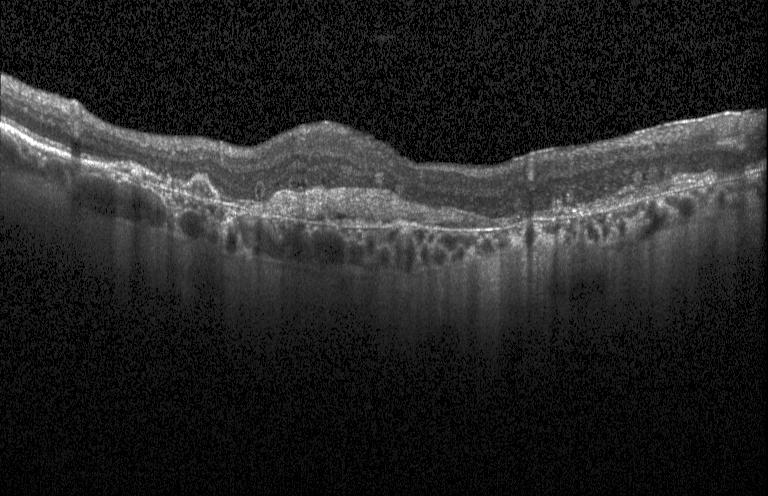 Optical coherence tomography scan.
This B-scan demonstrates choroidal neovascularization.